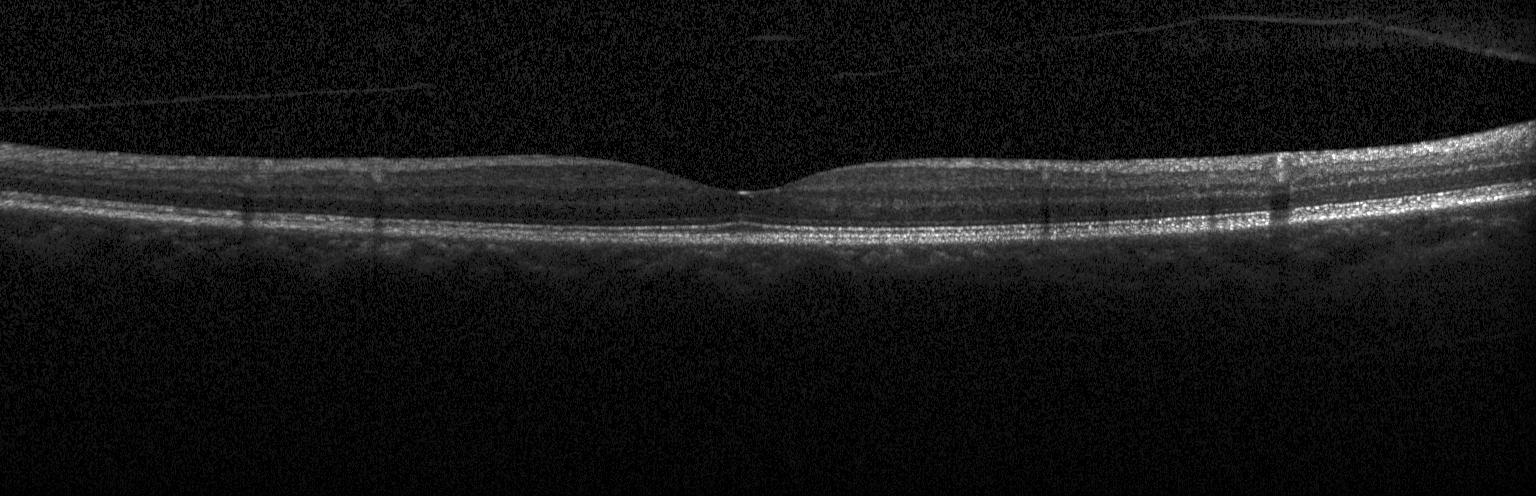
Heidelberg Spectralis OCT system; OCT line scan; horizontal scan through the fovea; spectral-domain OCT — Diagnosis: neither choroidal neovascularization, diabetic macular edema, nor drusen.